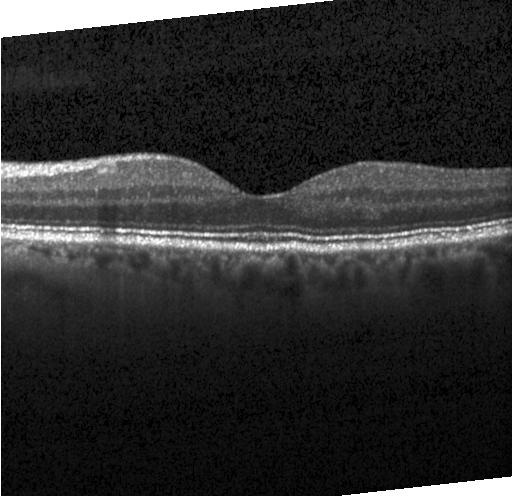

Assessment: no CNV, DME, or drusen.